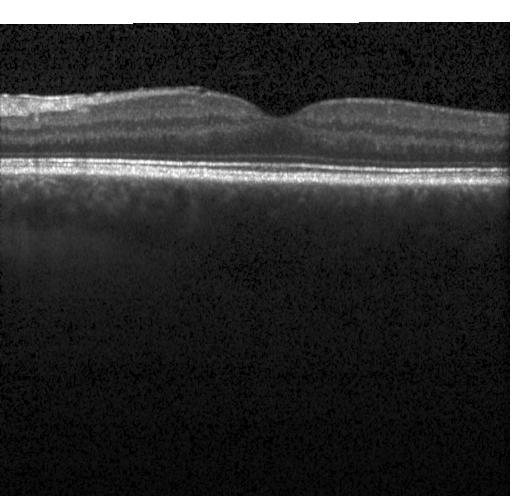
Acquired on a Heidelberg Spectralis. OCT B-scan. Fovea-centered. SD-OCT.
Impression: no choroidal neovascularization, diabetic macular edema, or drusen.